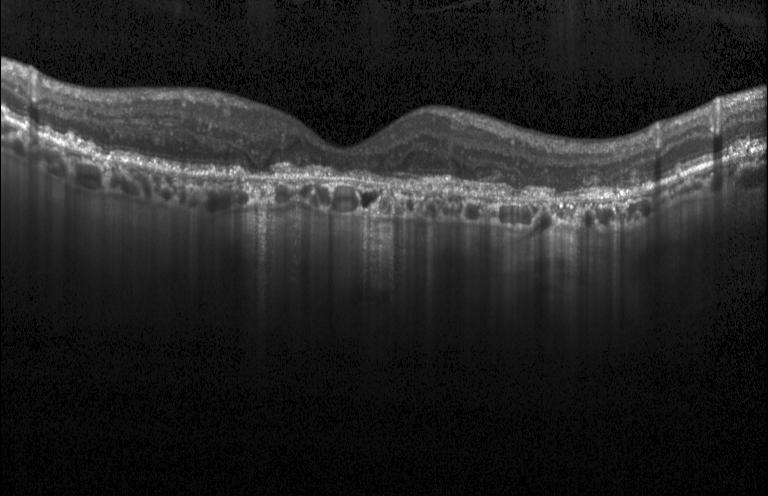 Instrument: Heidelberg Spectralis; spectral-domain OCT; retinal OCT B-scan
Dx: a choroidal neovascular membrane.